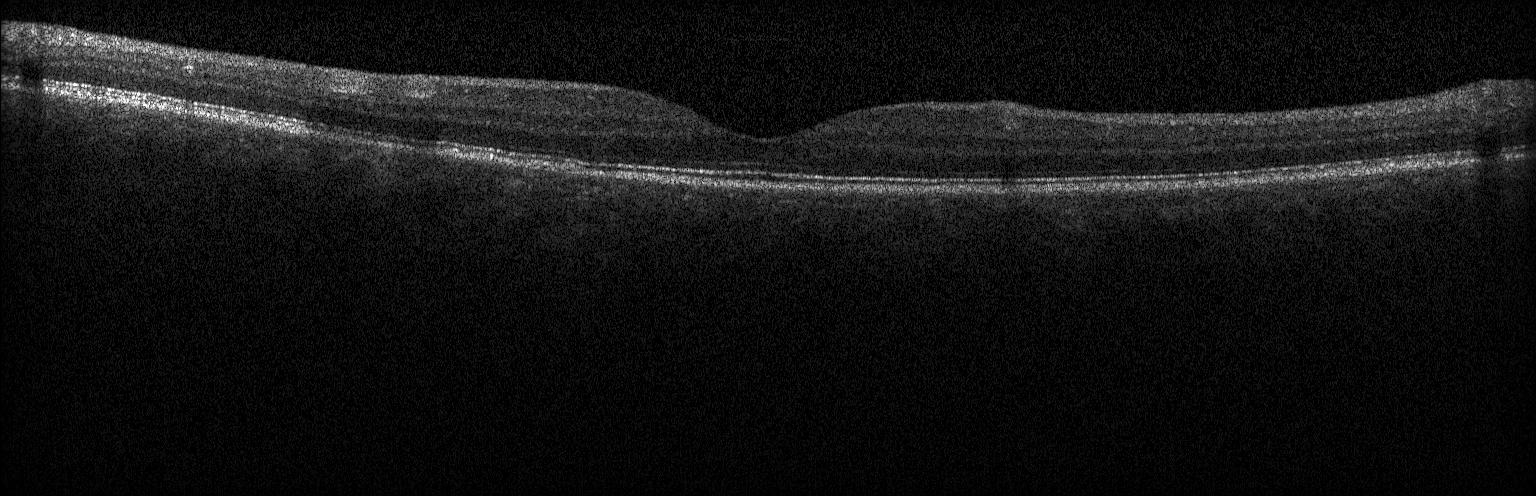

Optical coherence tomography B-scan
This B-scan demonstrates no choroidal neovascularization, no diabetic macular edema, and no drusen.